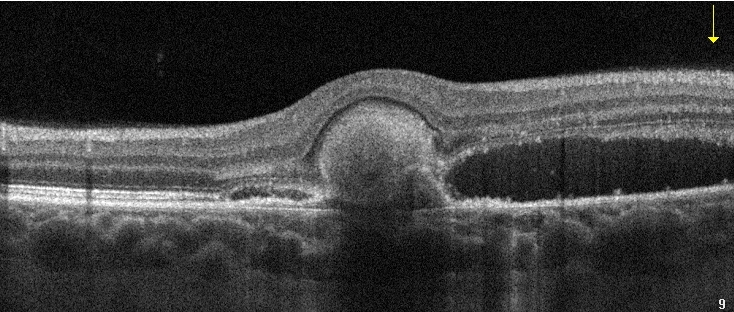

Optical coherence tomography B-scan.
Dx: AMD.